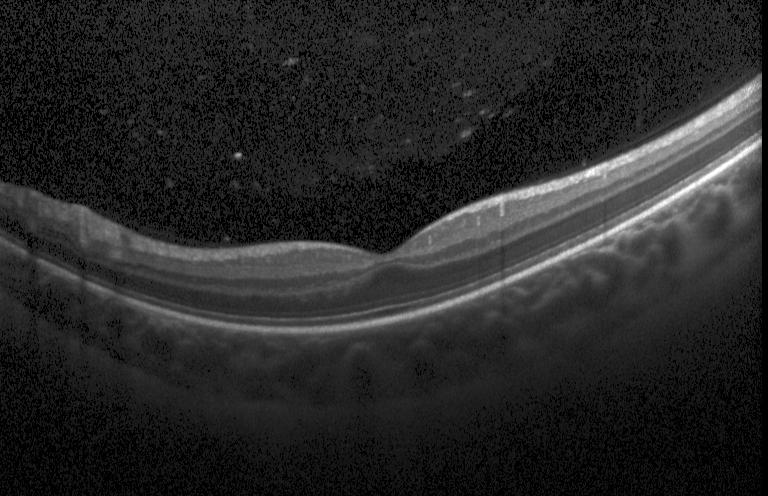

Fovea-centered, acquired on a Heidelberg Spectralis, OCT line scan, spectral-domain OCT
Finding: no choroidal neovascularization, diabetic macular edema, or drusen.